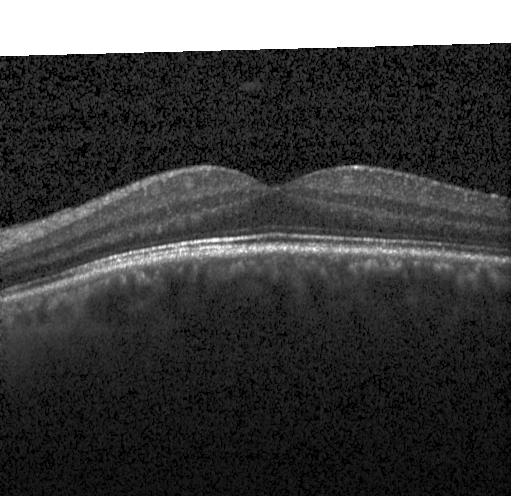 Optical coherence tomography scan. Neither CNV, DME, nor drusen.